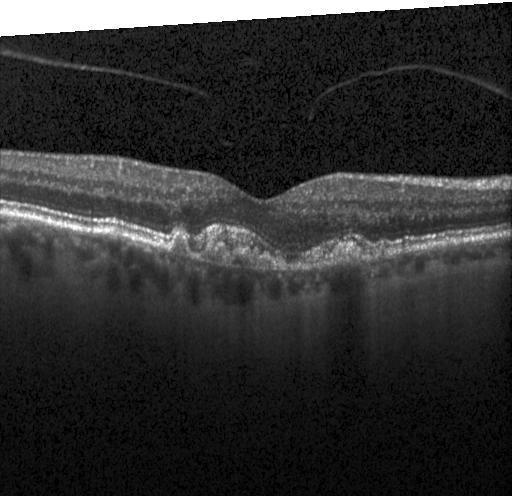 Impression: choroidal neovascularization (CNV).